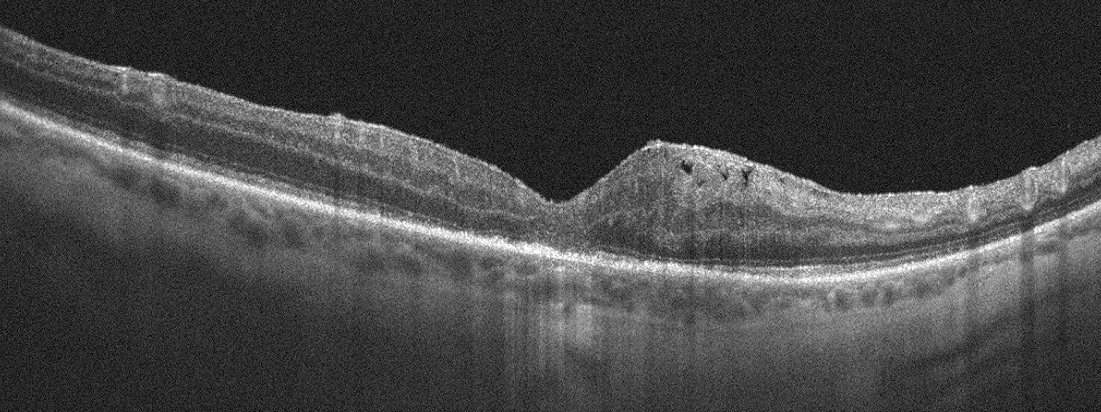
OCT scan showing diabetic macular edema (DME).